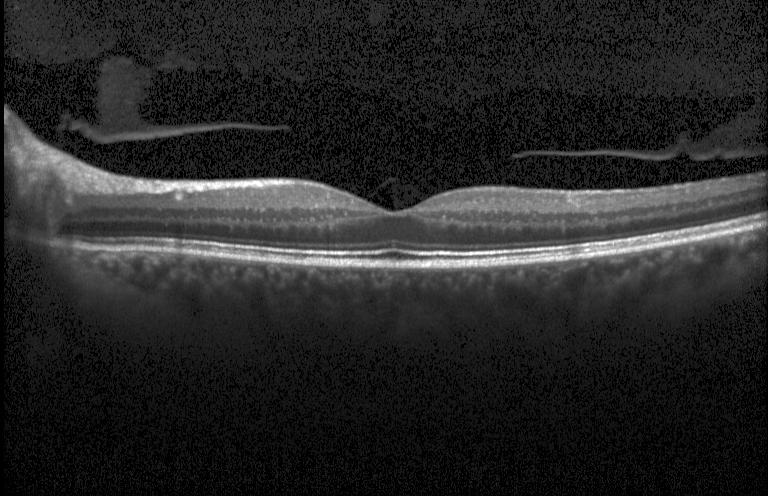 Spectral-domain optical coherence tomography; retinal OCT cross-section — Macular OCT: no choroidal neovascularization, no diabetic macular edema, and no drusen.